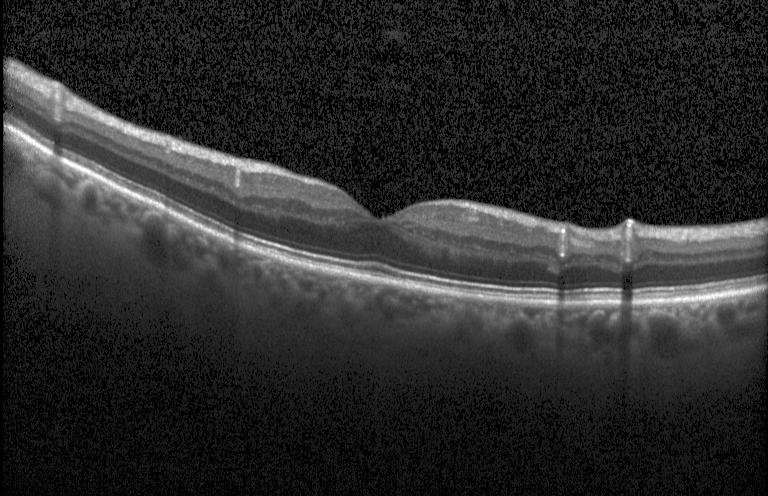 Diagnosis: neither choroidal neovascularization, diabetic macular edema, nor drusen.